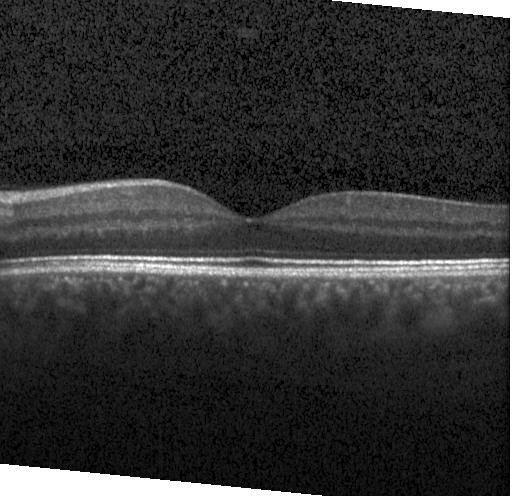

OCT B-scan showing no CNV, no DME, and no drusen.